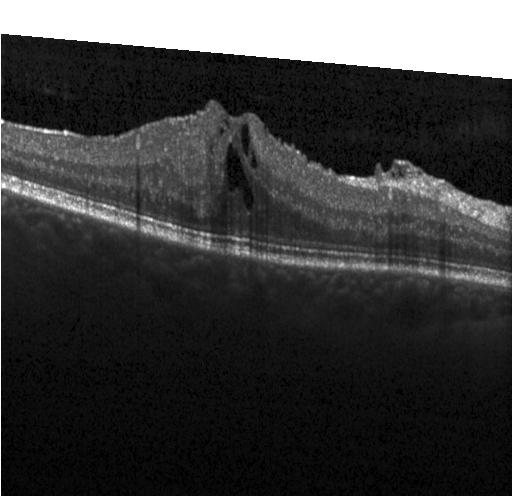

This B-scan demonstrates diabetic macular edema (DME).